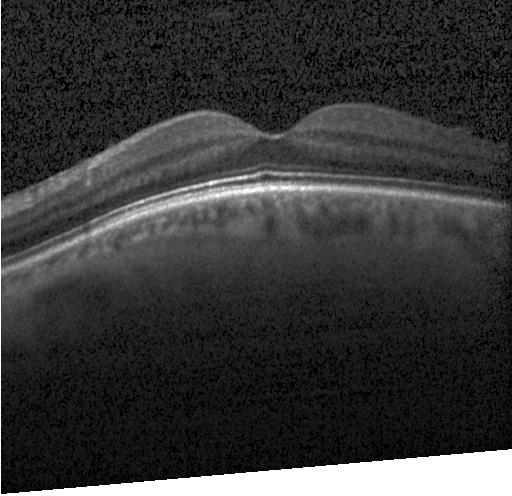

Macular scan. Spectral-domain OCT. Optical coherence tomography scan. Heidelberg Spectralis.
Diagnosis: no evidence of choroidal neovascularization, diabetic macular edema, or drusen.